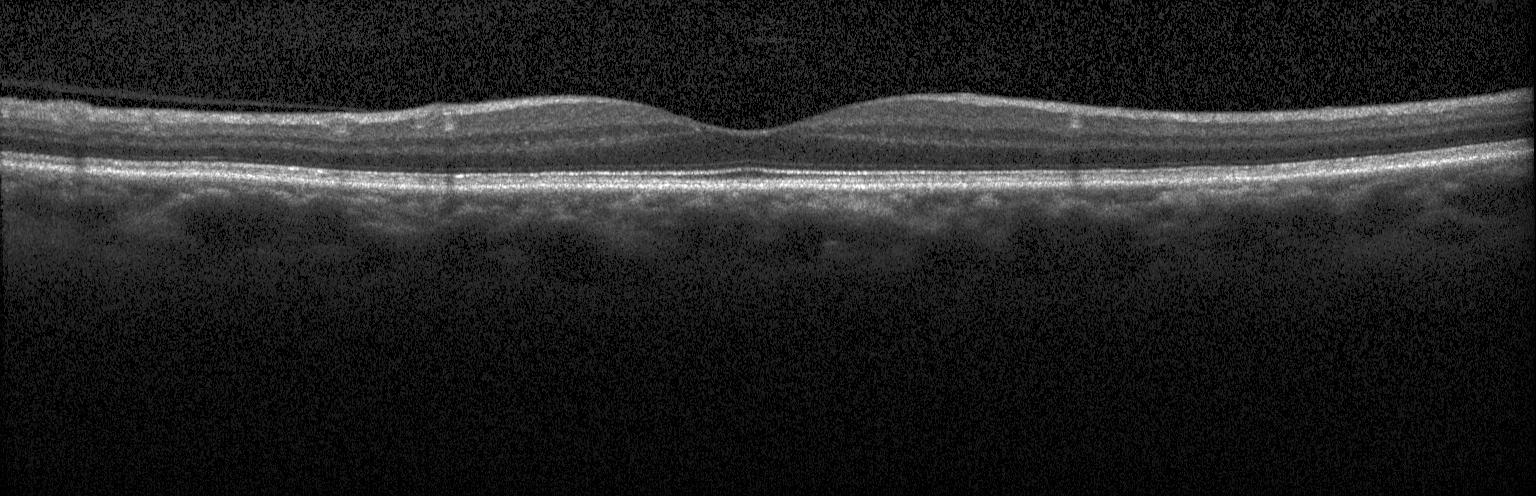

Finding: no CNV, DME, or drusen.